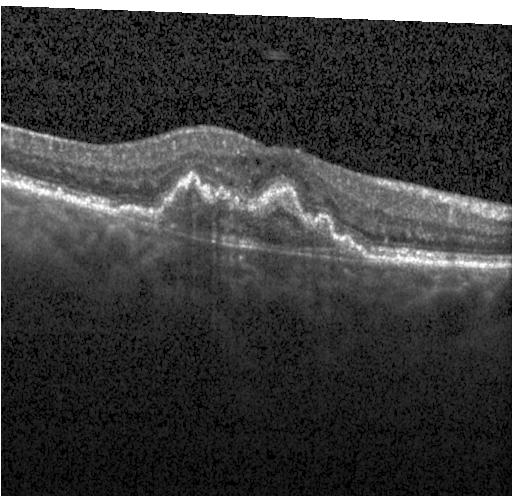

Heidelberg Spectralis; spectral-domain OCT; horizontal scan through the fovea; OCT B-scan.
Diagnosis: CNV.